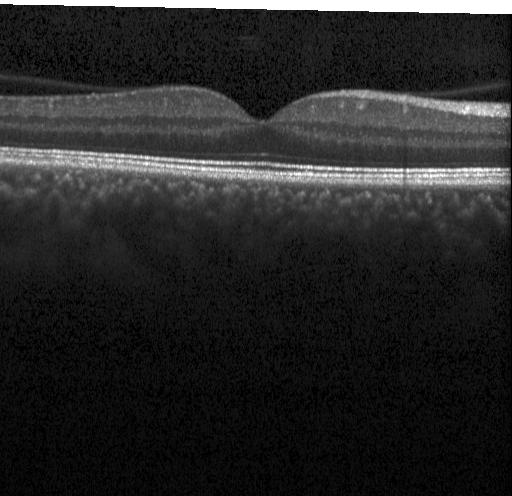

Diagnosis: neither CNV, DME, nor drusen.